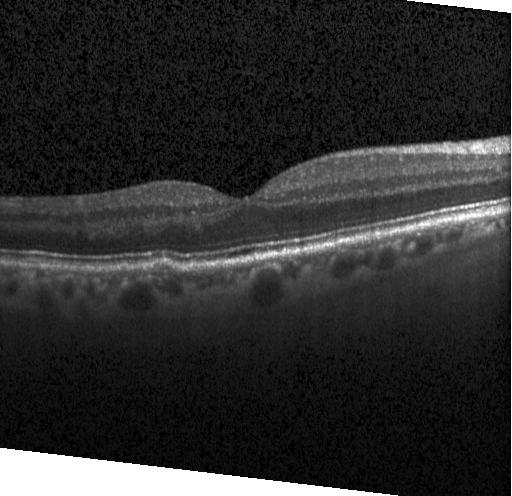
Retinal OCT cross-section. This B-scan demonstrates multiple drusen.